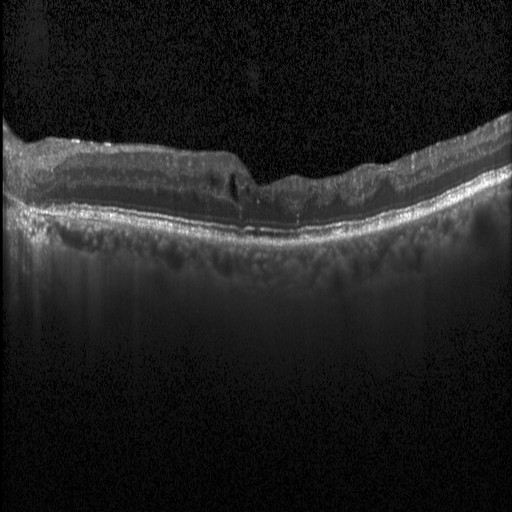 Finding: diabetic macular edema.